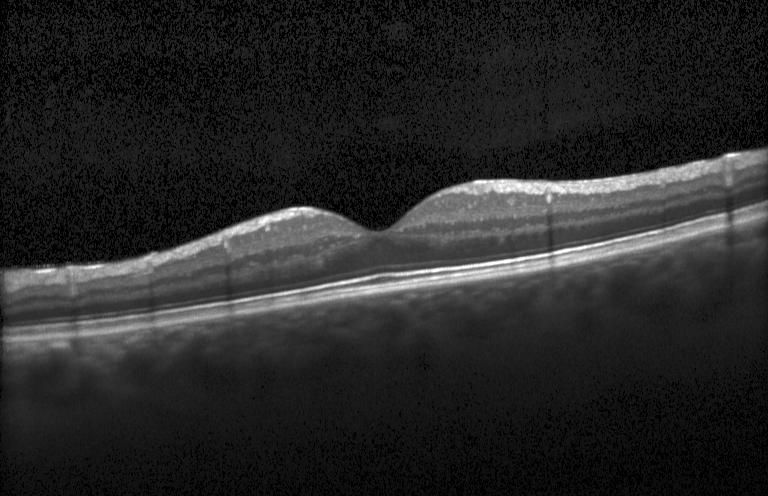

Heidelberg Spectralis OCT system, through the macula, OCT B-scan — Diagnosis: no evidence of choroidal neovascularization, diabetic macular edema, or drusen.